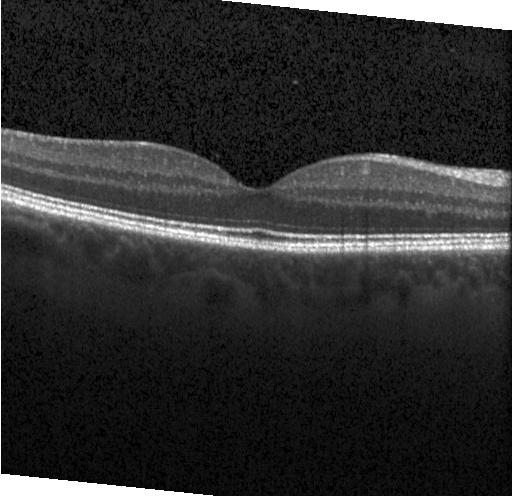
Retinal OCT B-scan
OCT finding: no evidence of CNV, DME, or drusen.